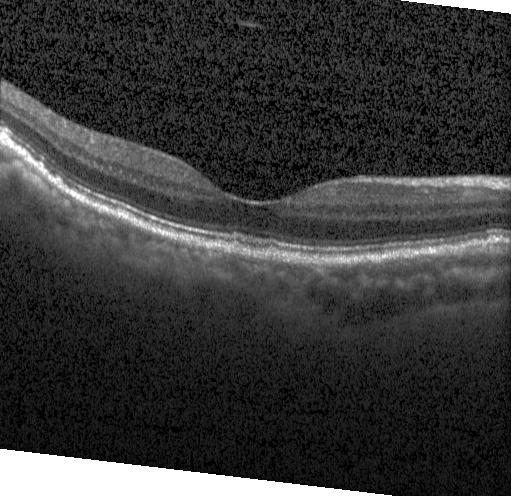
Optical coherence tomography scan · fovea-centered — Impression: no CNV, no DME, and no drusen.